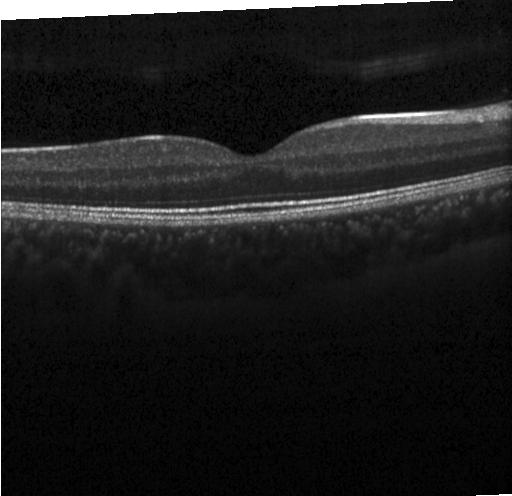 Macular OCT: no evidence of choroidal neovascularization, diabetic macular edema, or drusen.